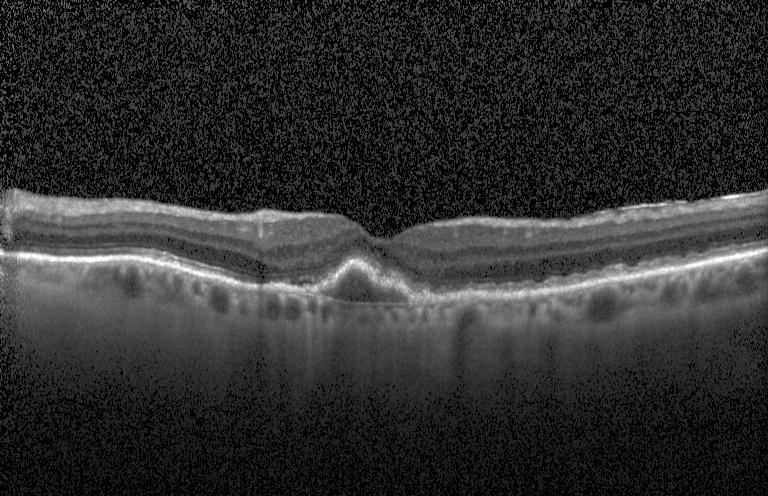
Optical coherence tomography scan. The scan shows a choroidal neovascular membrane.